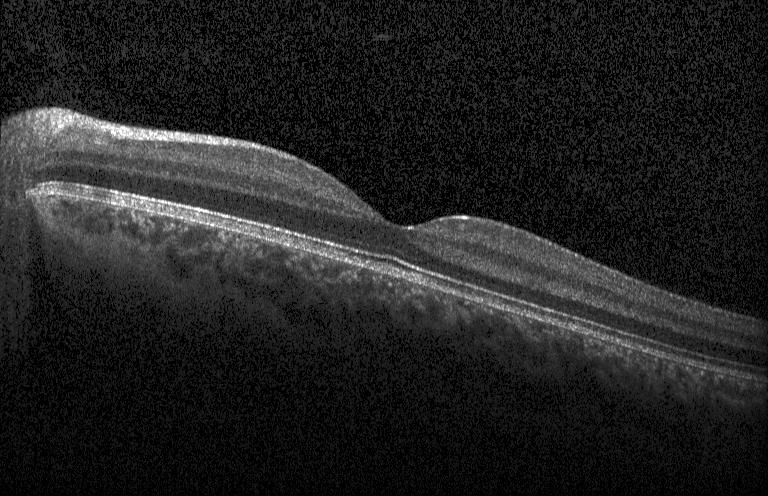

OCT line scan; spectral-domain OCT; fovea-centered.
Finding: neither CNV, DME, nor drusen.